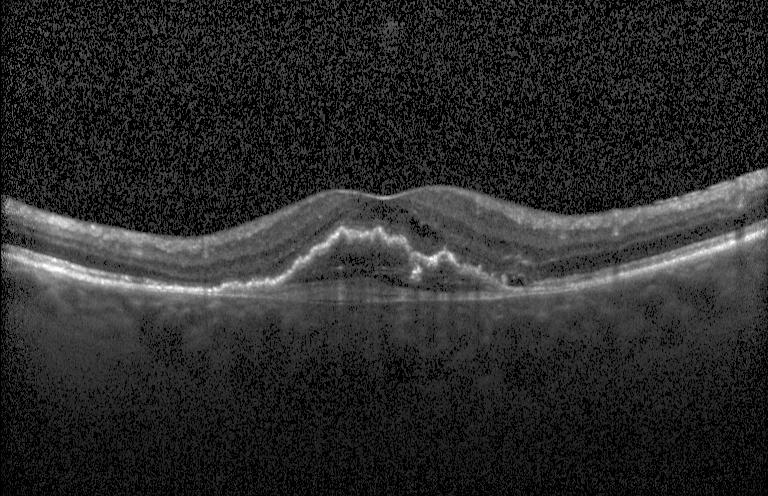
Impression: choroidal neovascularization (CNV).